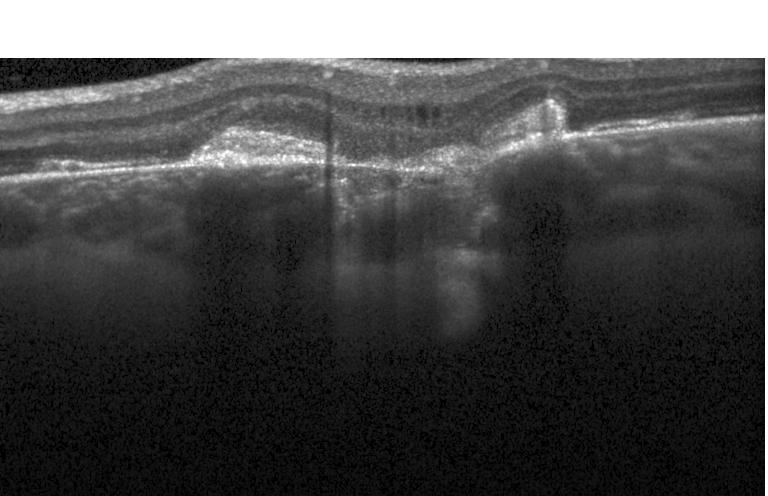
Macular OCT: choroidal neovascularization.